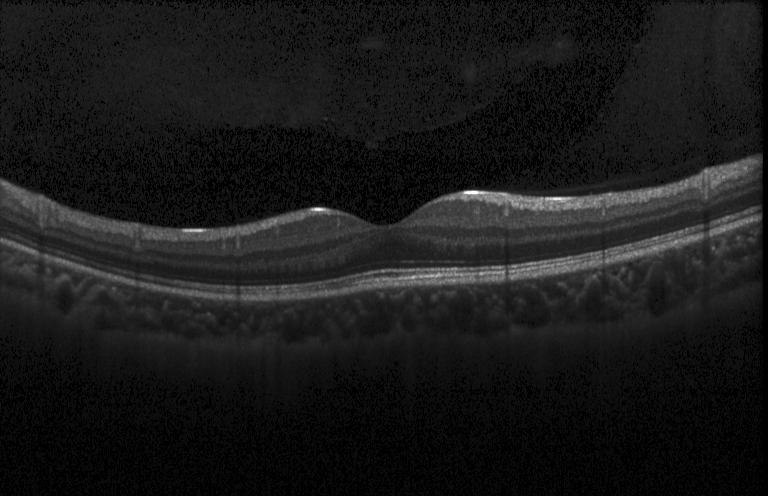 Retinal OCT cross-section; SD-OCT. Macular OCT: no evidence of choroidal neovascularization, diabetic macular edema, or drusen.